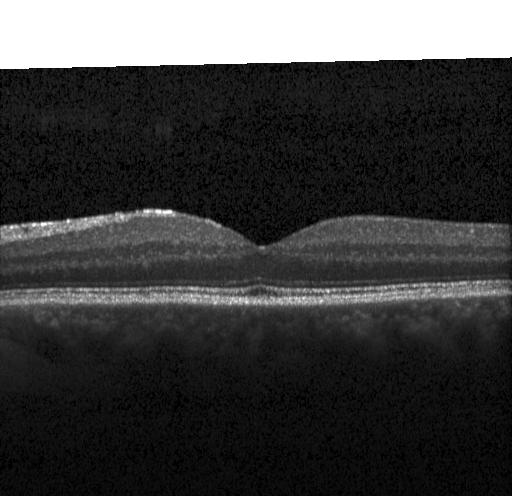
No choroidal neovascularization, diabetic macular edema, or drusen.